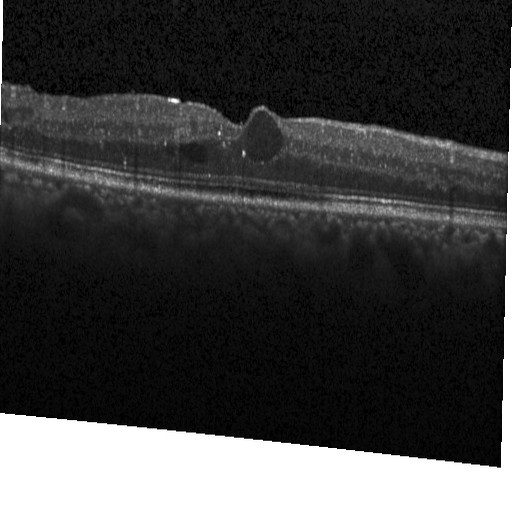
Horizontal scan through the fovea · optical coherence tomography scan · Heidelberg Spectralis
Impression: DME.